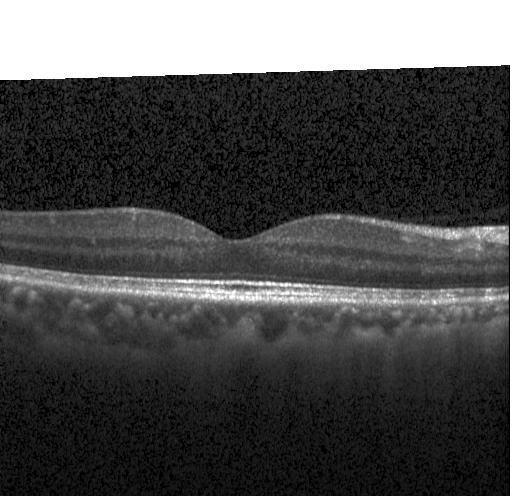

Heidelberg Spectralis · horizontal scan through the fovea · OCT B-scan — Diagnosis: neither CNV, DME, nor drusen.